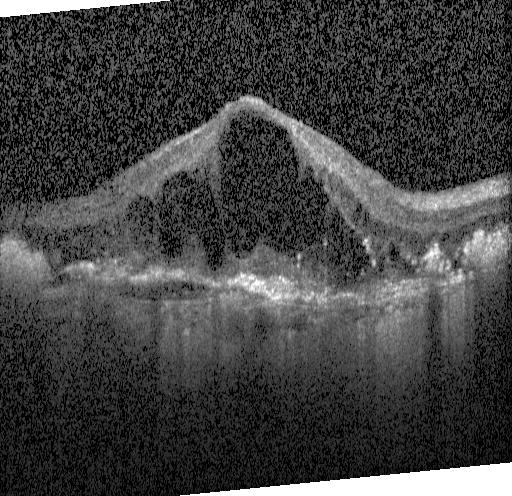 This B-scan demonstrates a choroidal neovascular membrane.